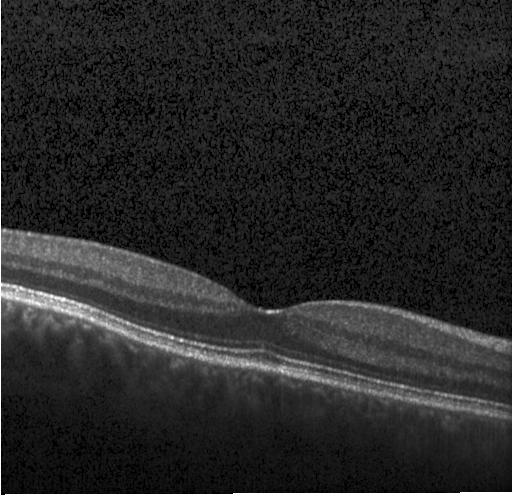
Impression: no evidence of choroidal neovascularization, diabetic macular edema, or drusen.